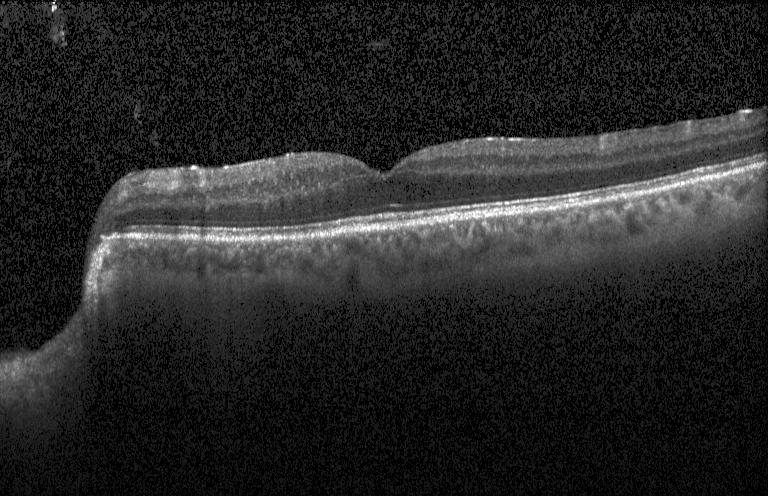
Instrument: Heidelberg Spectralis; macular scan; OCT line scan — The scan shows neither choroidal neovascularization, diabetic macular edema, nor drusen.